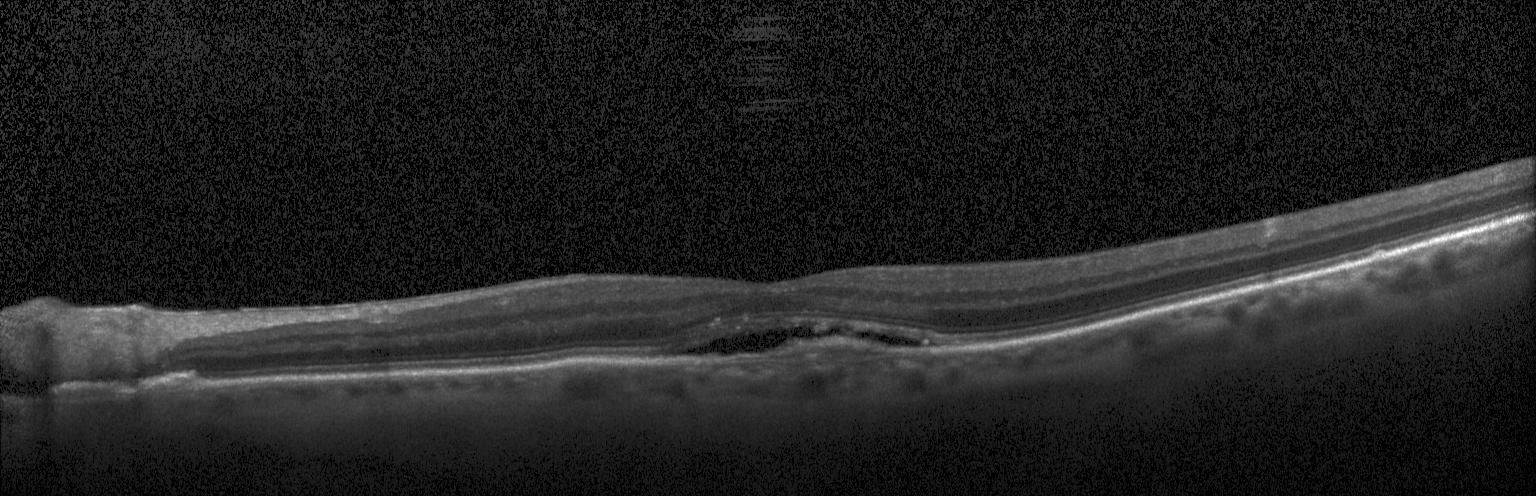

Optical coherence tomography B-scan.
Assessment: CNV.